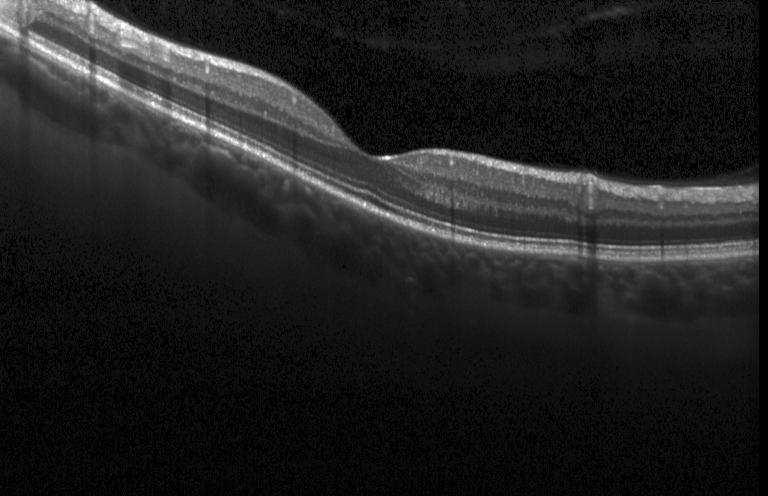
SD-OCT · fovea-centered · OCT B-scan · instrument: Heidelberg Spectralis.
Macular OCT: neither CNV, DME, nor drusen.